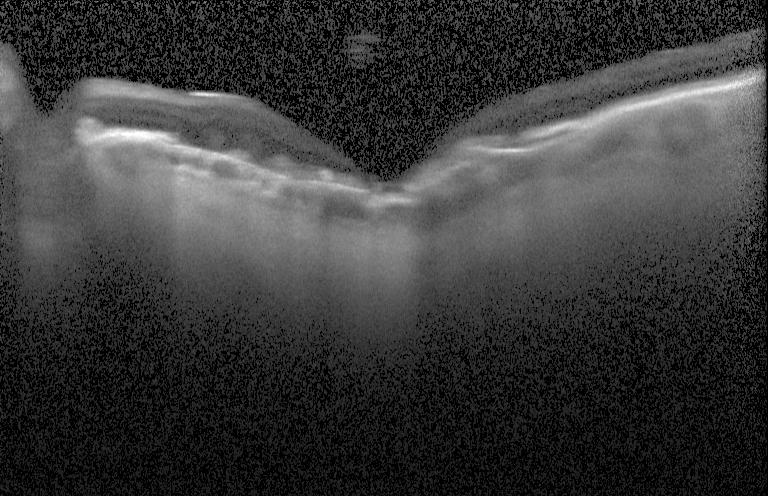

Optical coherence tomography B-scan. This B-scan demonstrates a choroidal neovascular membrane.